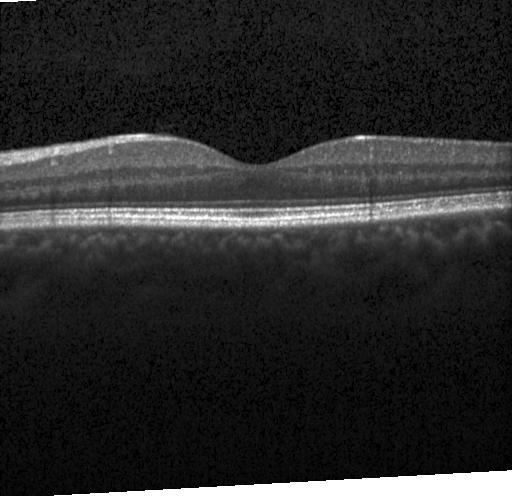
Spectral-domain optical coherence tomography. Through the macula. OCT line scan. Instrument: Heidelberg Spectralis. This B-scan demonstrates no CNV, no DME, and no drusen.